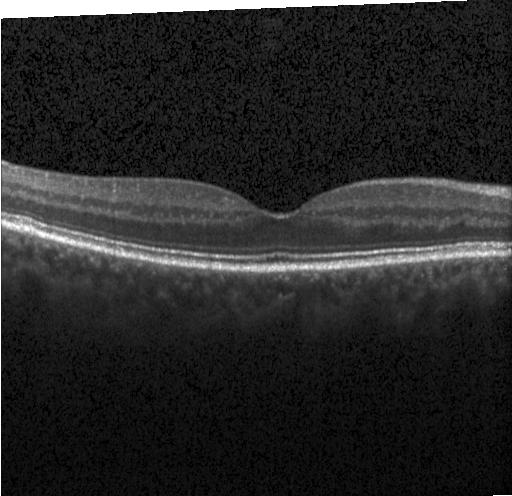 Macular OCT demonstrating no choroidal neovascularization, no diabetic macular edema, and no drusen.